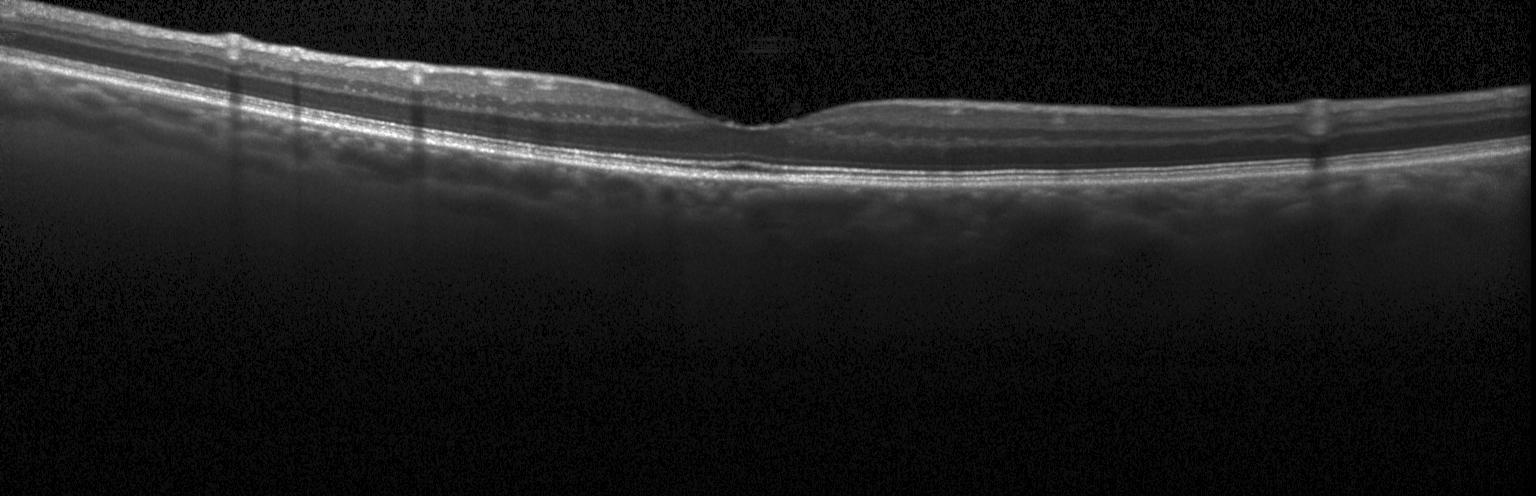

SD-OCT · retinal OCT B-scan. Finding: neither choroidal neovascularization, diabetic macular edema, nor drusen.